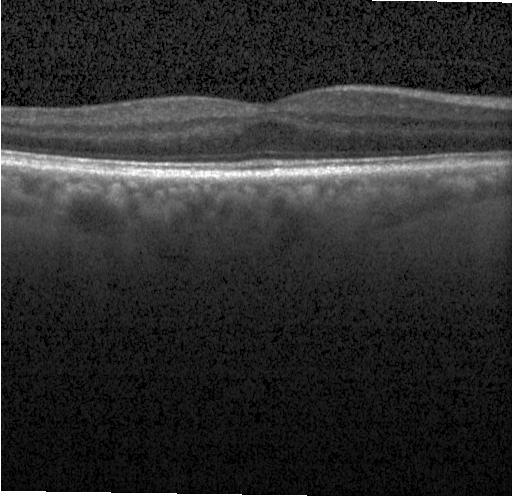

OCT line scan; spectral-domain OCT; acquired on a Heidelberg Spectralis.
Assessment: no evidence of CNV, DME, or drusen.